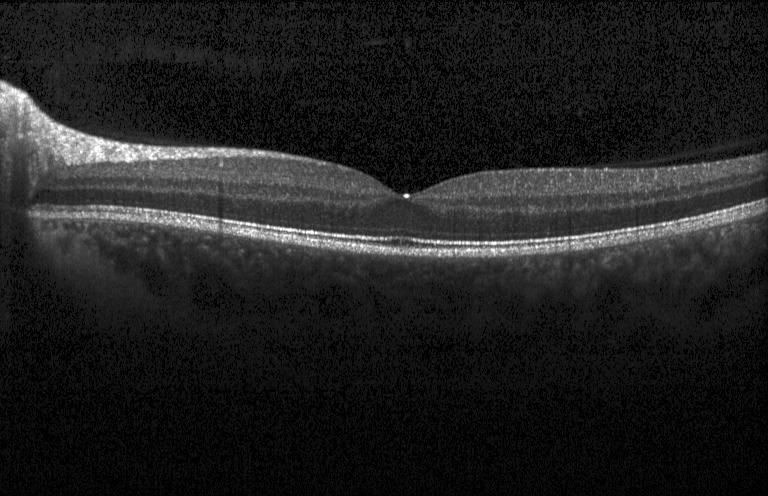 Finding: no choroidal neovascularization, diabetic macular edema, or drusen.